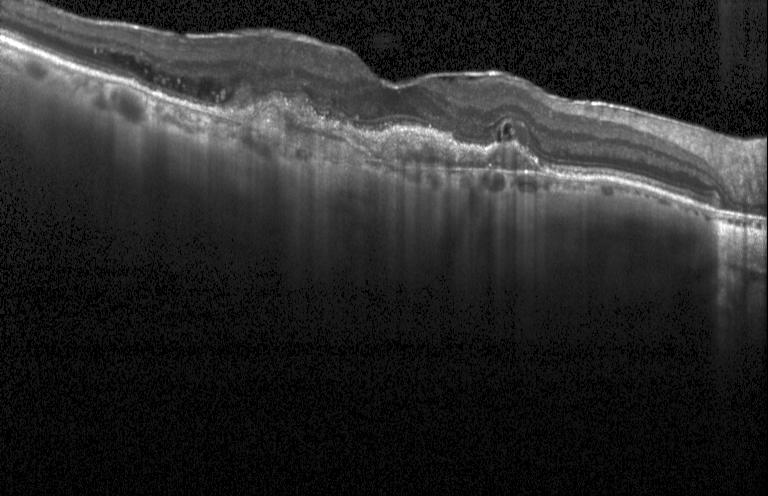 Spectral-domain optical coherence tomography, optical coherence tomography scan.
Diagnosis: CNV.